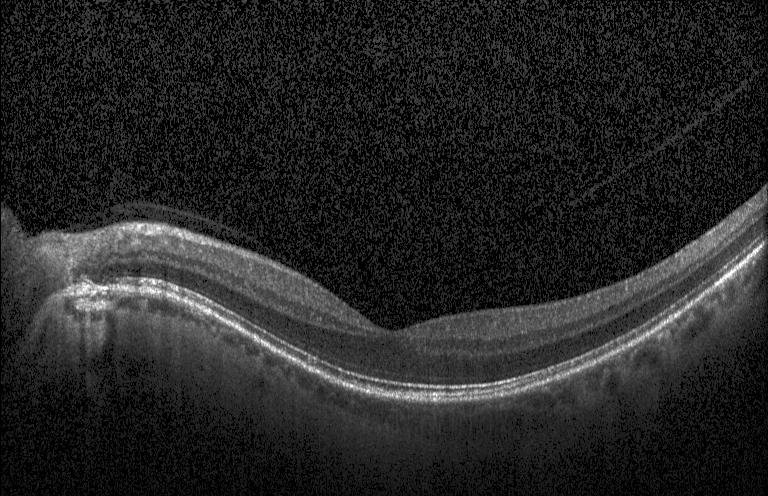
Spectral-domain OCT B-scan: no choroidal neovascularization, diabetic macular edema, or drusen.